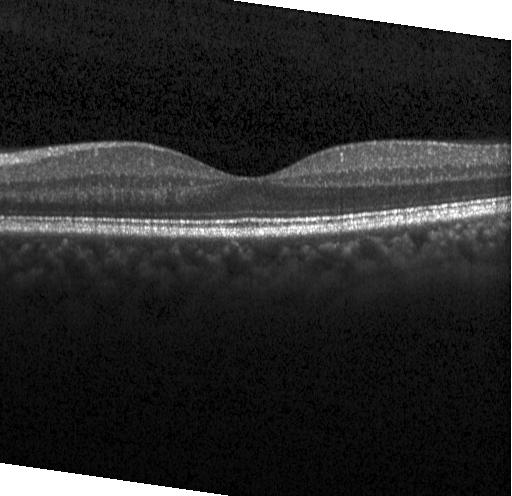
Optical coherence tomography B-scan — Finding: neither choroidal neovascularization, diabetic macular edema, nor drusen.